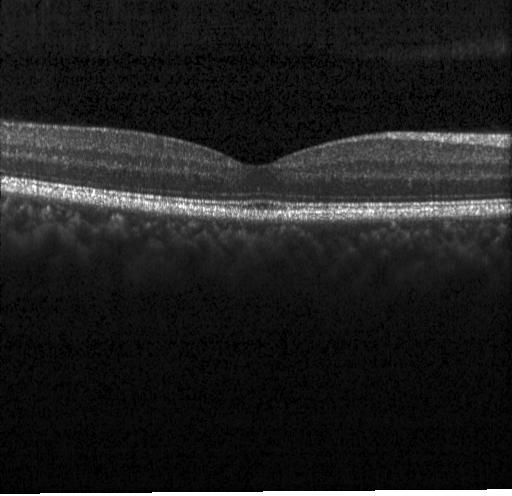

Optical coherence tomography scan
Impression: no evidence of choroidal neovascularization, diabetic macular edema, or drusen.